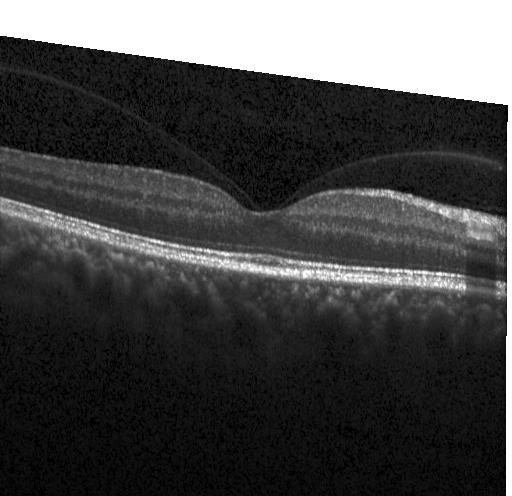 Horizontal scan through the fovea; SD-OCT; optical coherence tomography B-scan.
Macular OCT: no choroidal neovascularization, diabetic macular edema, or drusen.